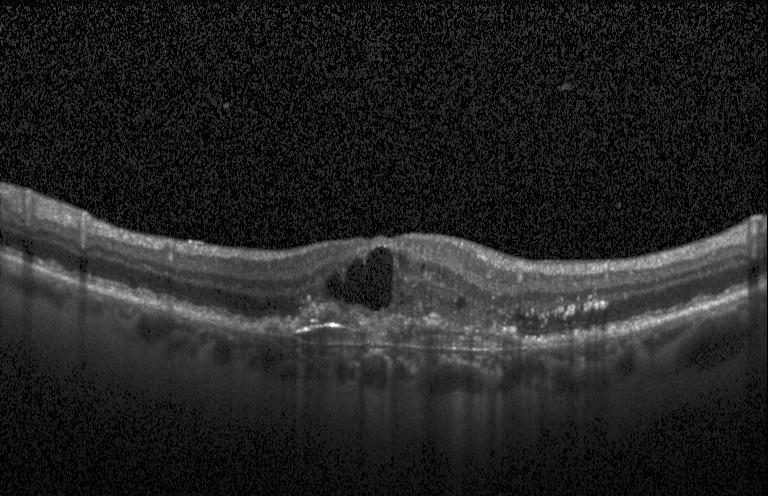

OCT B-scan; macular scan; Heidelberg Spectralis OCT system.
Dx: a choroidal neovascular membrane.